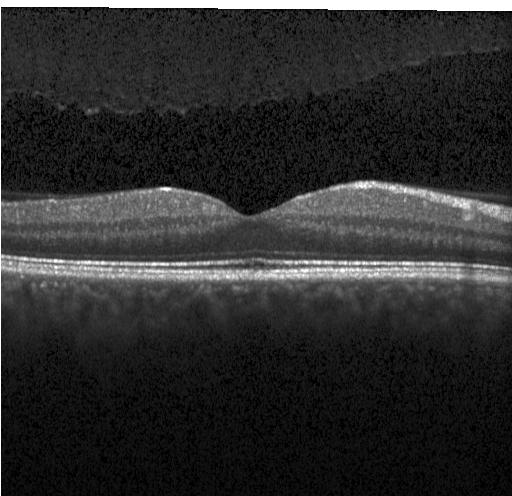 Optical coherence tomography scan; spectral-domain OCT.
This B-scan demonstrates no choroidal neovascularization, no diabetic macular edema, and no drusen.